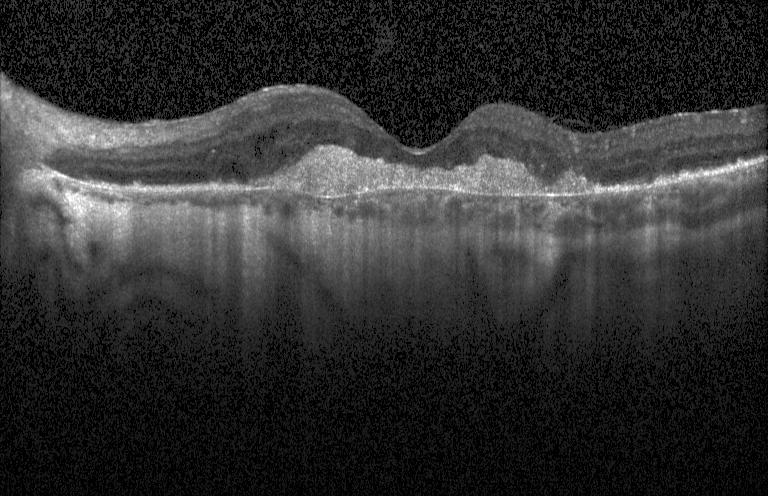

Macular OCT demonstrating choroidal neovascularization.